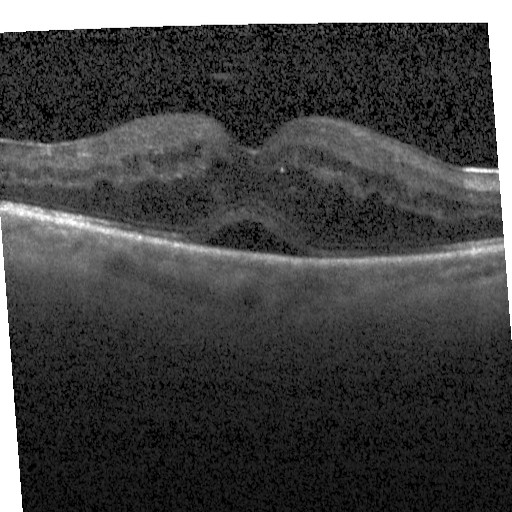 Optical coherence tomography scan · through the macula · SD-OCT · Heidelberg Spectralis — The scan shows diabetic macular edema.